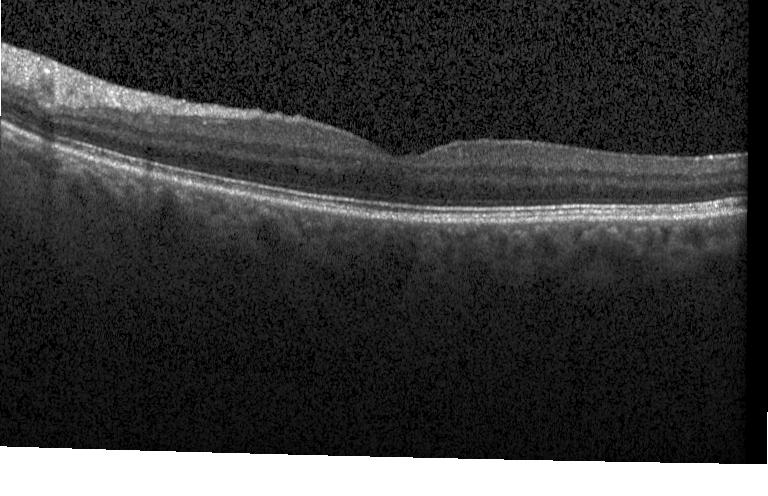
Centered on the fovea · retinal OCT B-scan · acquired on a Heidelberg Spectralis — No evidence of CNV, DME, or drusen.